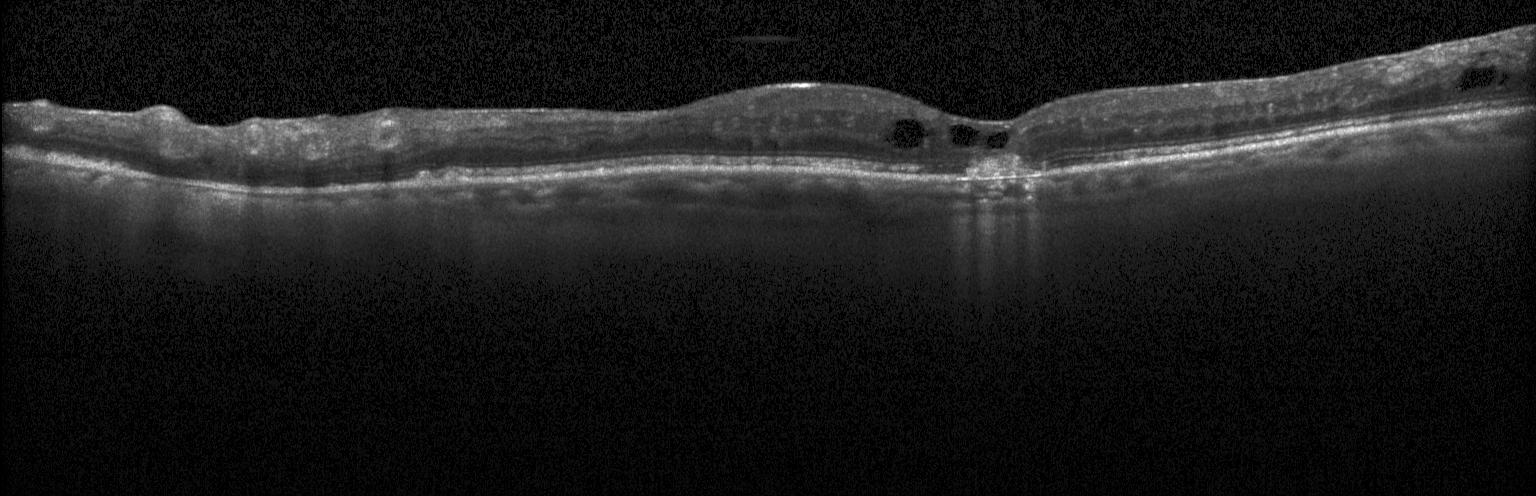
Heidelberg Spectralis OCT system, optical coherence tomography scan, spectral-domain OCT, horizontal scan through the fovea
The scan shows a choroidal neovascular membrane.